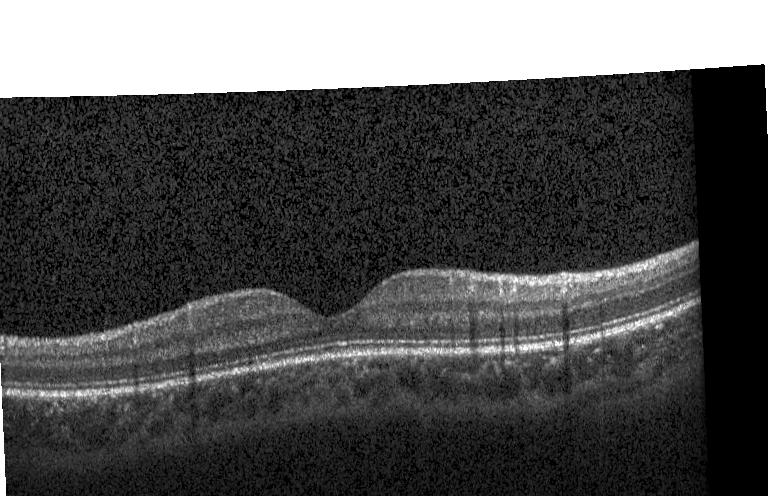

Optical coherence tomography scan · spectral-domain optical coherence tomography · Heidelberg Spectralis.
Macular OCT: no CNV, no DME, and no drusen.